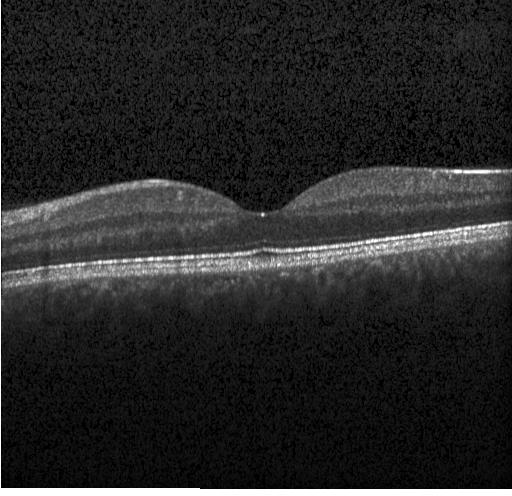 Spectral-domain OCT · optical coherence tomography B-scan
OCT finding: no choroidal neovascularization, no diabetic macular edema, and no drusen.